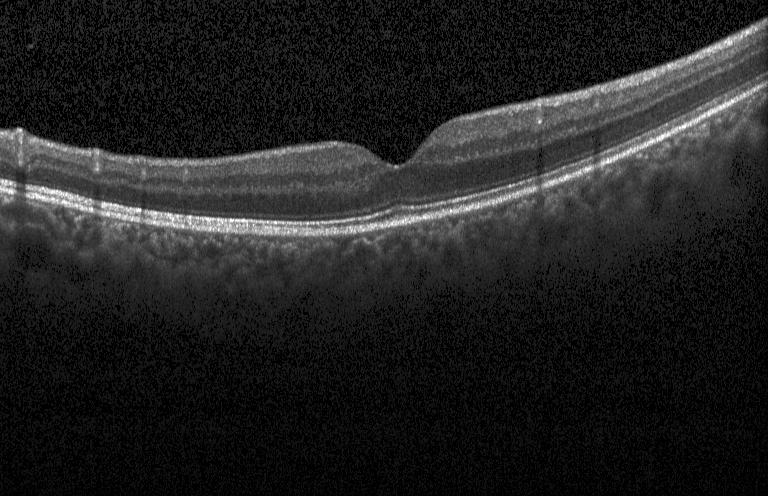
Assessment: neither choroidal neovascularization, diabetic macular edema, nor drusen.